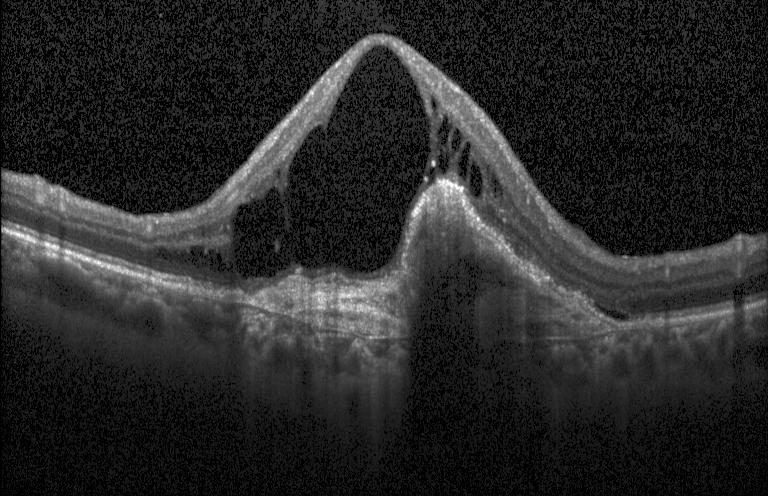
Diagnosis: a choroidal neovascular membrane.